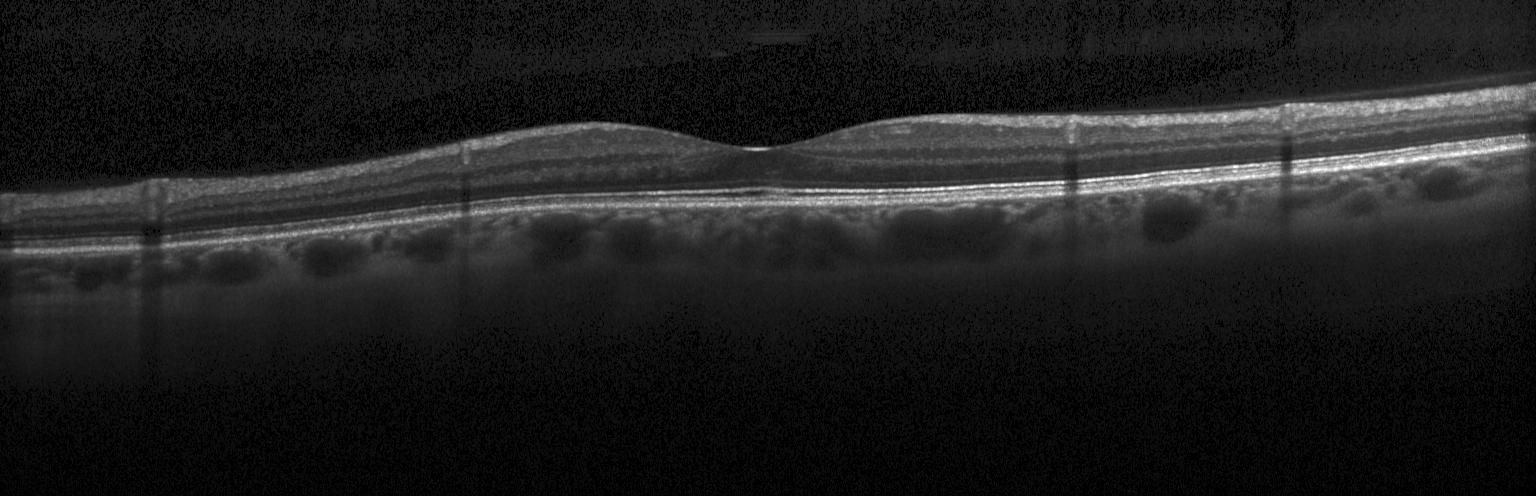 Retinal OCT B-scan — Macular OCT: neither choroidal neovascularization, diabetic macular edema, nor drusen.